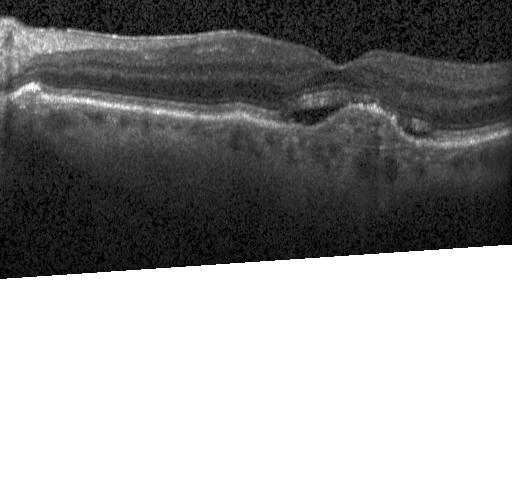 This B-scan demonstrates a choroidal neovascular membrane.